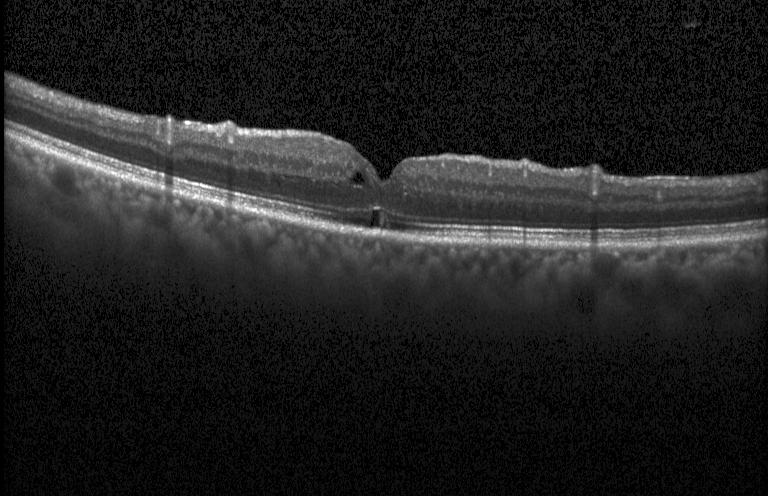

OCT scan showing diabetic macular edema (DME).